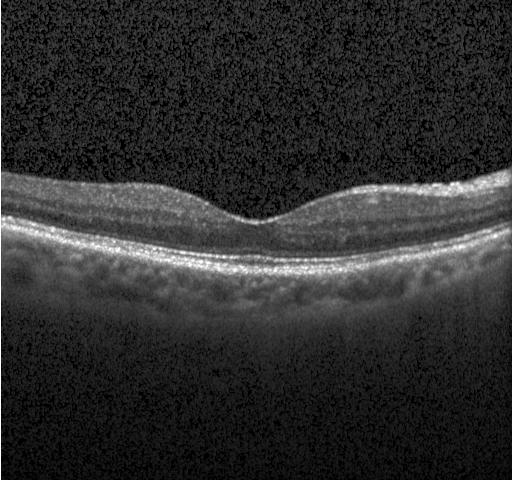
Retinal OCT cross-section; fovea-centered; SD-OCT. Dx: no evidence of choroidal neovascularization, diabetic macular edema, or drusen.